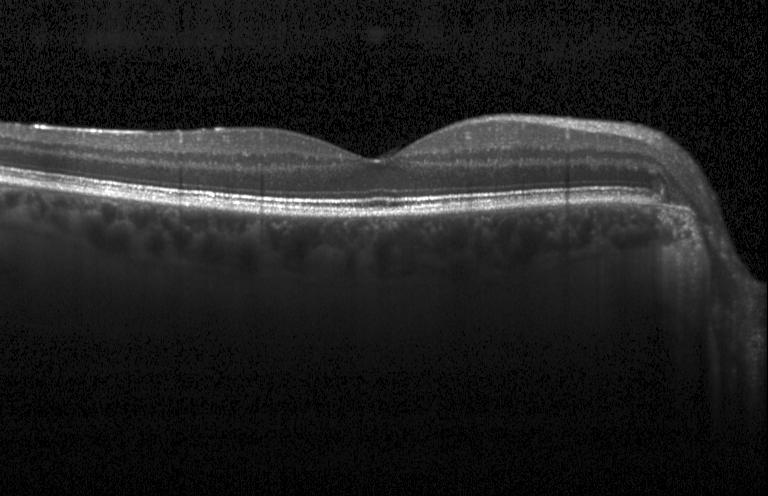
Horizontal scan through the fovea. Retinal OCT B-scan. SD-OCT. Impression: no choroidal neovascularization, diabetic macular edema, or drusen.